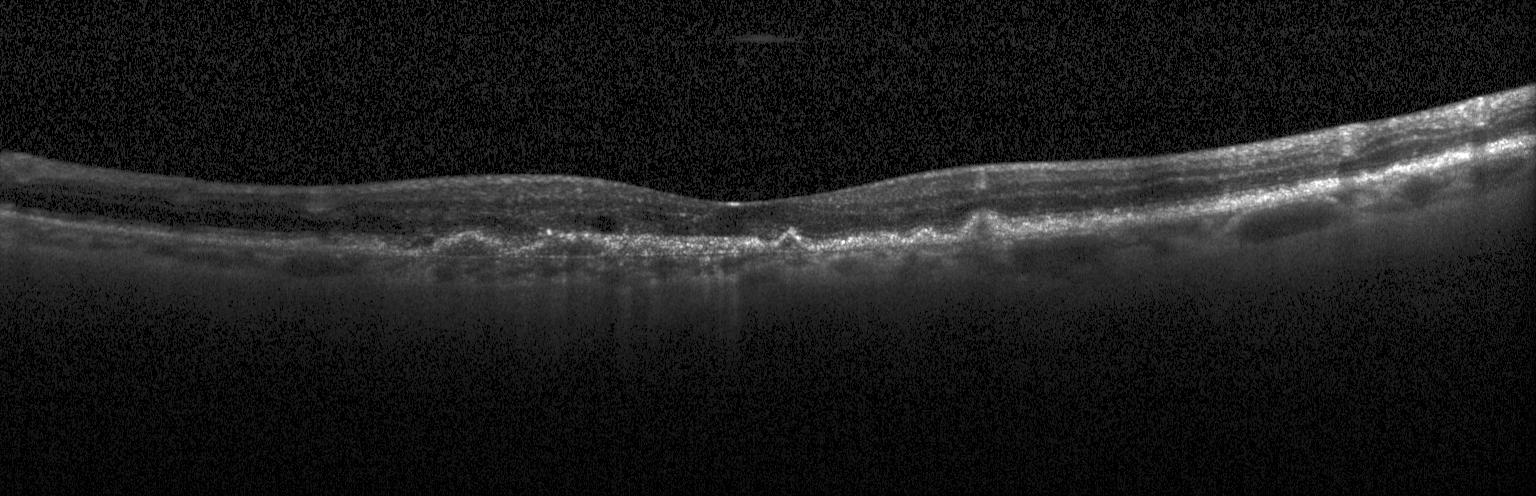 Impression: CNV.